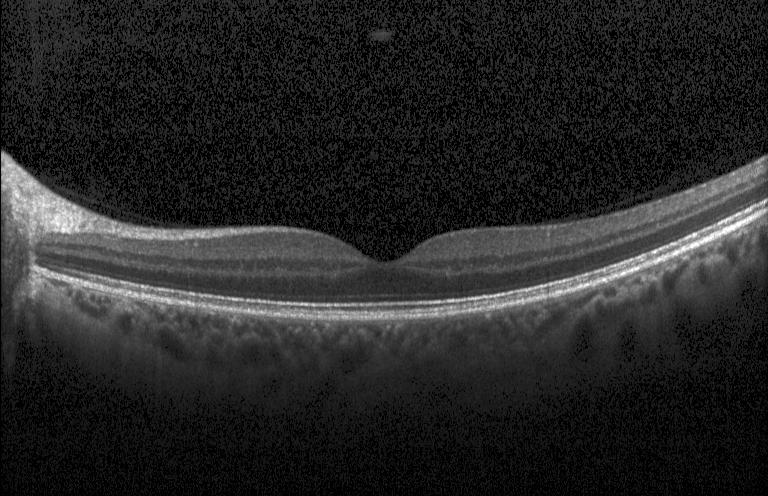

Acquired on a Heidelberg Spectralis. OCT line scan. Macular scan. Spectral-domain optical coherence tomography
This B-scan demonstrates neither choroidal neovascularization, diabetic macular edema, nor drusen.